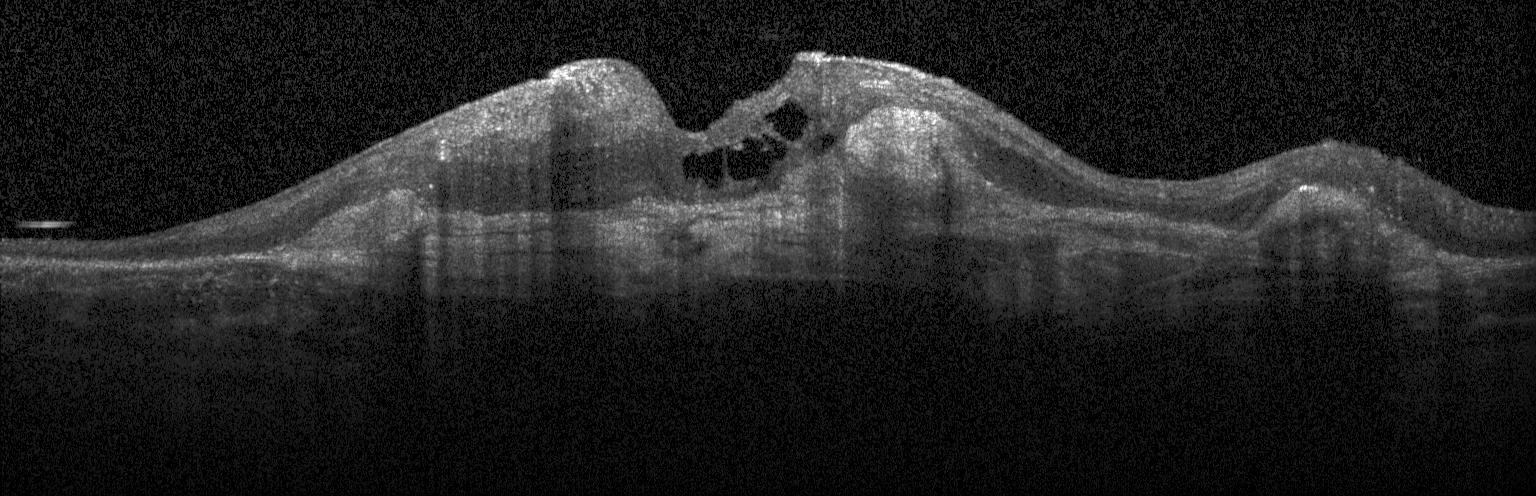
OCT B-scan showing a choroidal neovascular membrane.